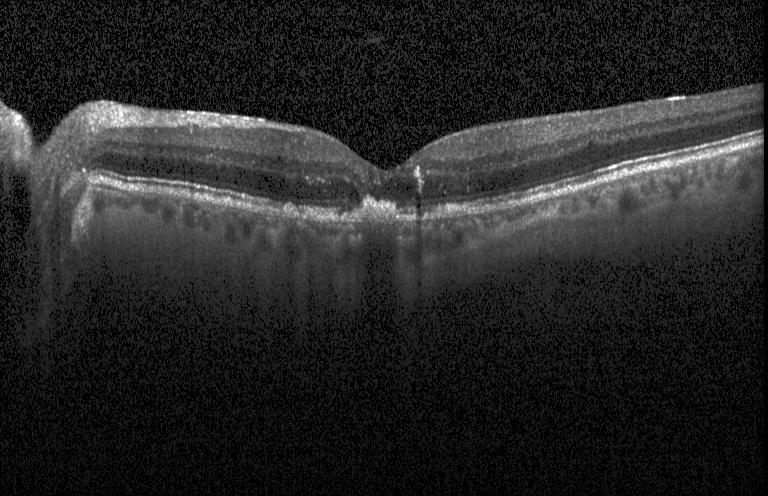

Retinal OCT B-scan · horizontal scan through the fovea · spectral-domain optical coherence tomography — OCT finding: a choroidal neovascular membrane.